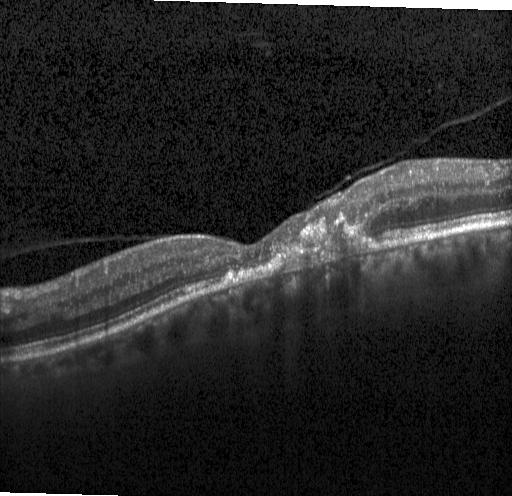 Spectral-domain optical coherence tomography. Through the macula. Heidelberg Spectralis OCT system. Optical coherence tomography scan
This B-scan demonstrates CNV.